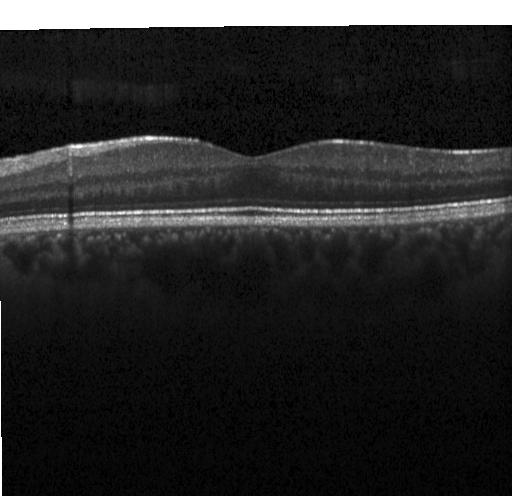

Spectral-domain OCT; fovea-centered; Heidelberg Spectralis; optical coherence tomography B-scan. This B-scan demonstrates no evidence of CNV, DME, or drusen.